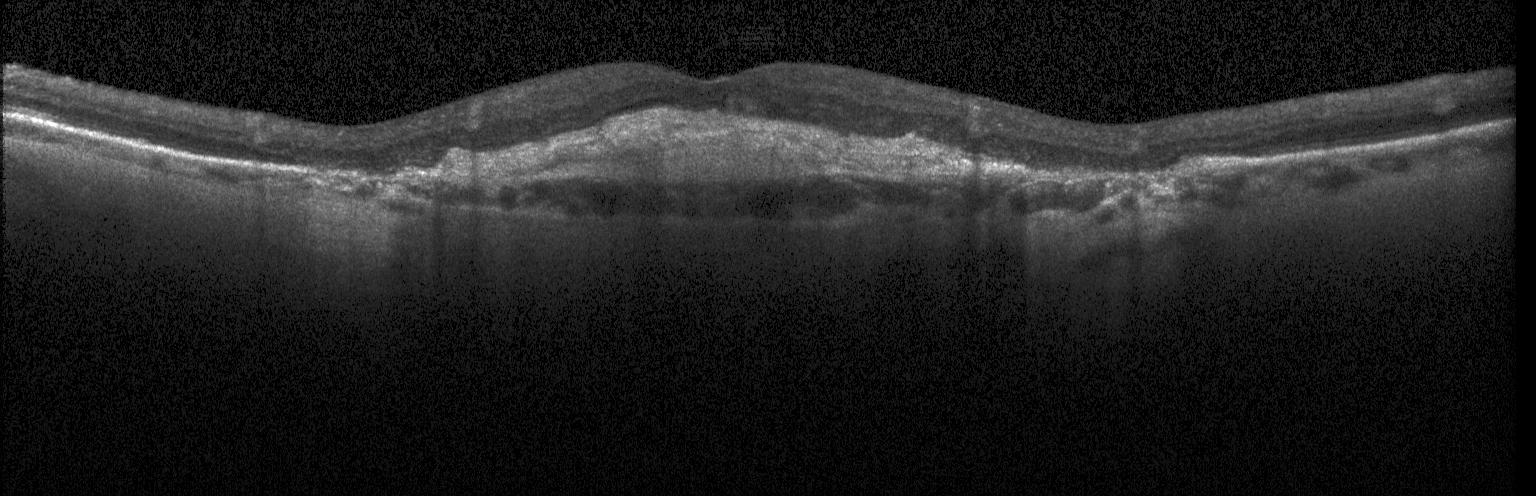

Retinal OCT B-scan. OCT finding: a choroidal neovascular membrane.